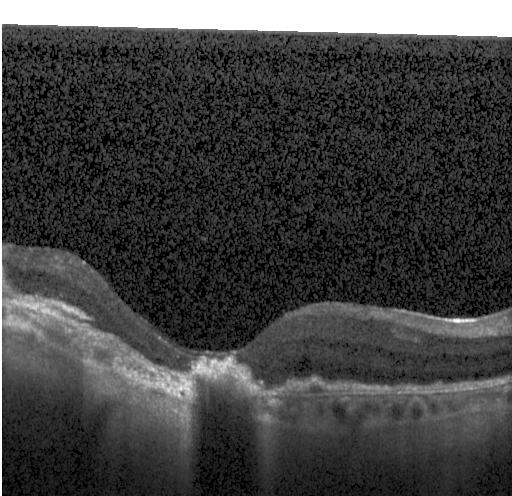 Retinal OCT cross-section showing a choroidal neovascular membrane.